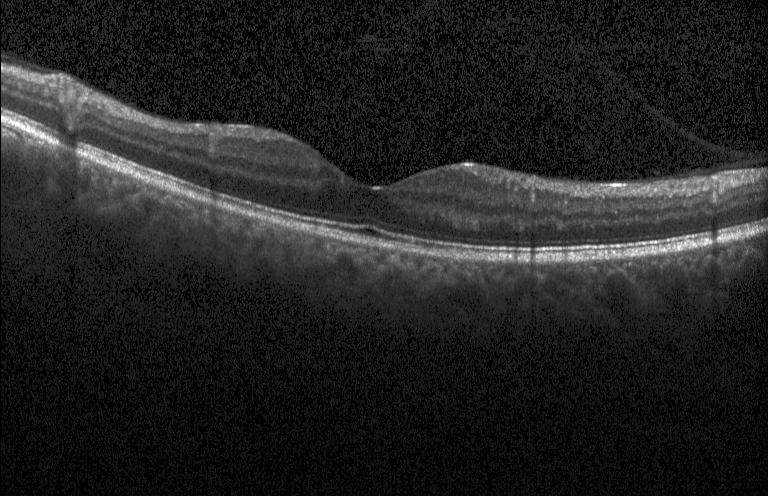
SD-OCT · optical coherence tomography B-scan — Diagnosis: no CNV, DME, or drusen.